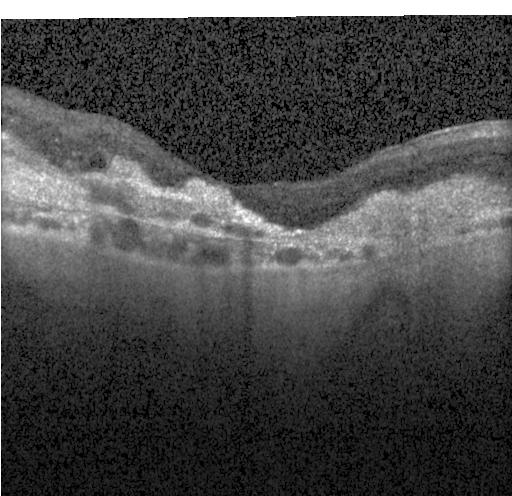 Centered on the fovea, optical coherence tomography scan, SD-OCT, acquired on a Heidelberg Spectralis. Finding: choroidal neovascularization.